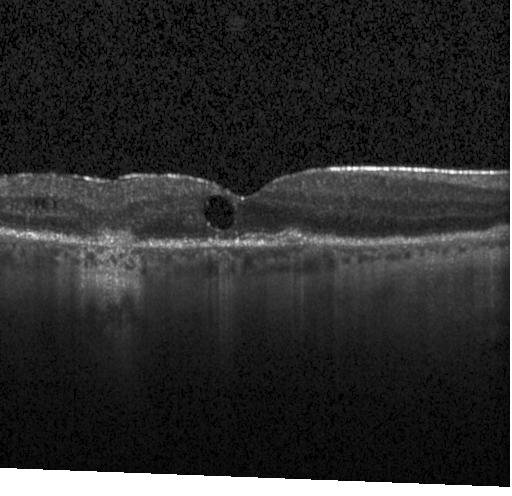 Impression: a choroidal neovascular membrane.